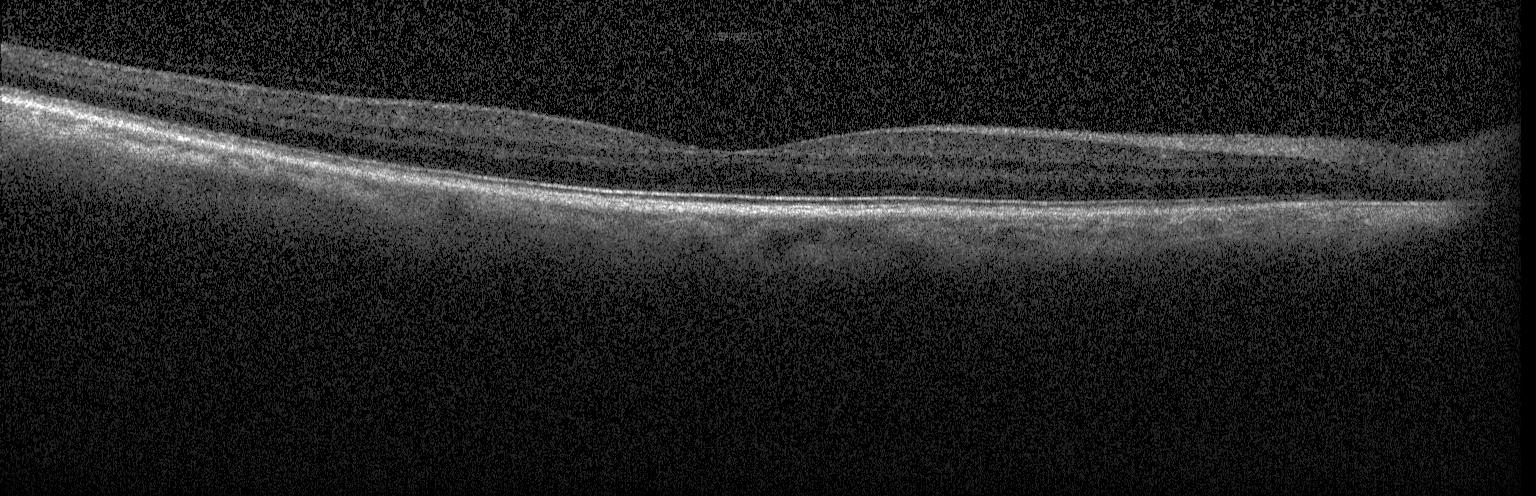 Optical coherence tomography scan — Diagnosis: no evidence of choroidal neovascularization, diabetic macular edema, or drusen.